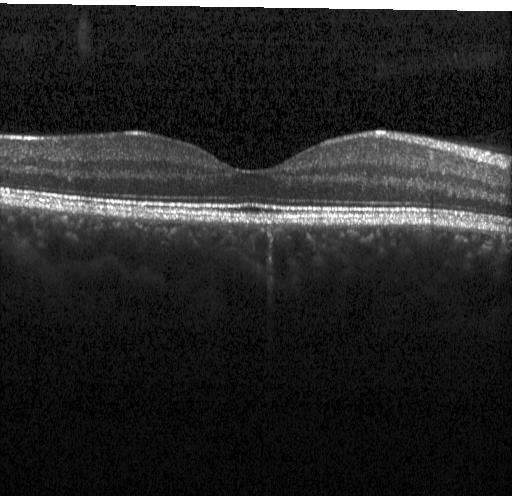 Retinal OCT cross-section — Diagnosis: no evidence of choroidal neovascularization, diabetic macular edema, or drusen.